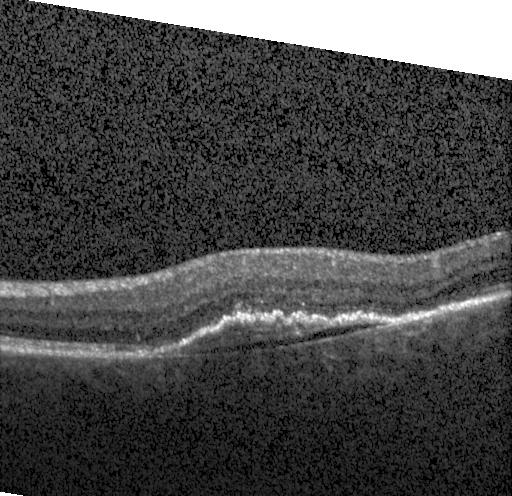

Retinal OCT cross-section showing a choroidal neovascular membrane.